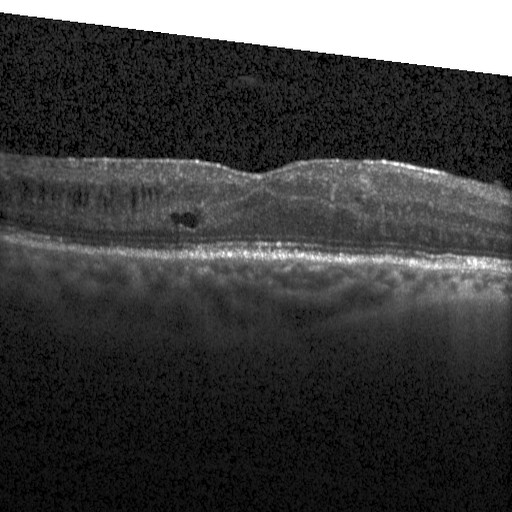
Optical coherence tomography scan · instrument: Heidelberg Spectralis.
Impression: DME.